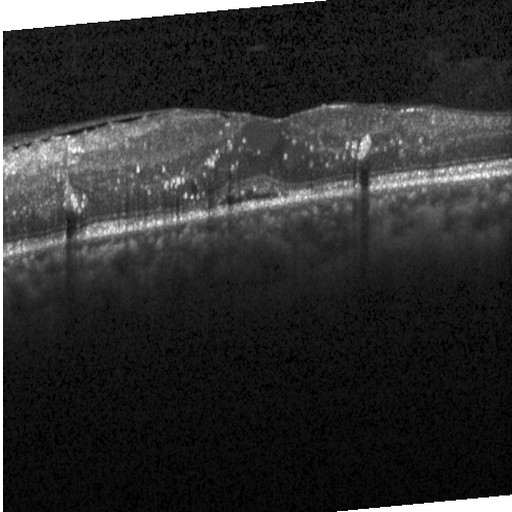 Spectral-domain OCT B-scan: diabetic macular edema.